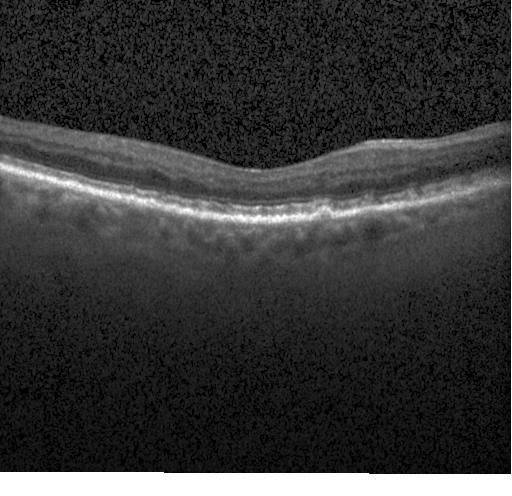

Retinal OCT cross-section, Heidelberg Spectralis. Assessment: drusen.